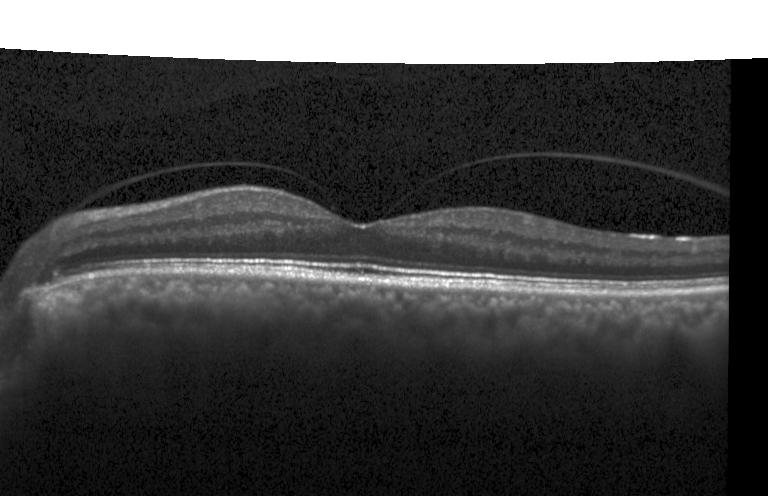 Spectral-domain optical coherence tomography. OCT line scan. Acquired on a Heidelberg Spectralis. Centered on the fovea — Assessment: neither choroidal neovascularization, diabetic macular edema, nor drusen.